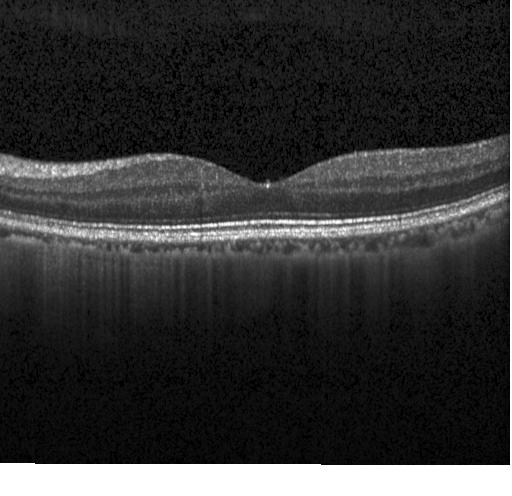

Optical coherence tomography scan
This B-scan demonstrates no choroidal neovascularization, no diabetic macular edema, and no drusen.